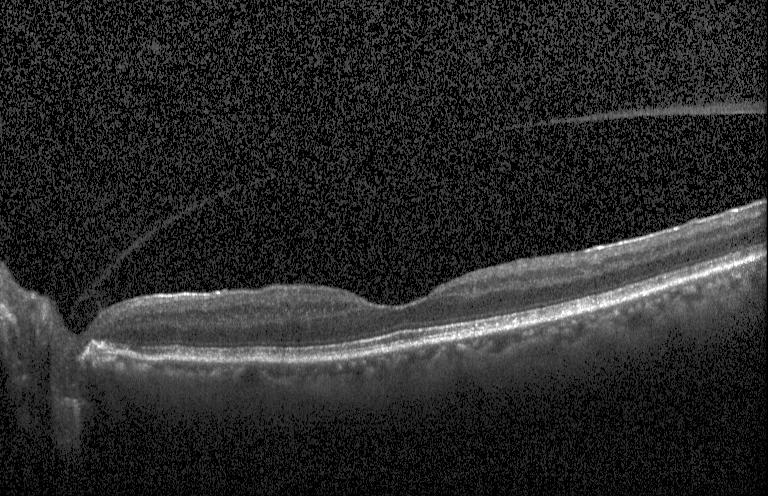 Instrument: Heidelberg Spectralis · optical coherence tomography scan
OCT finding: no evidence of choroidal neovascularization, diabetic macular edema, or drusen.